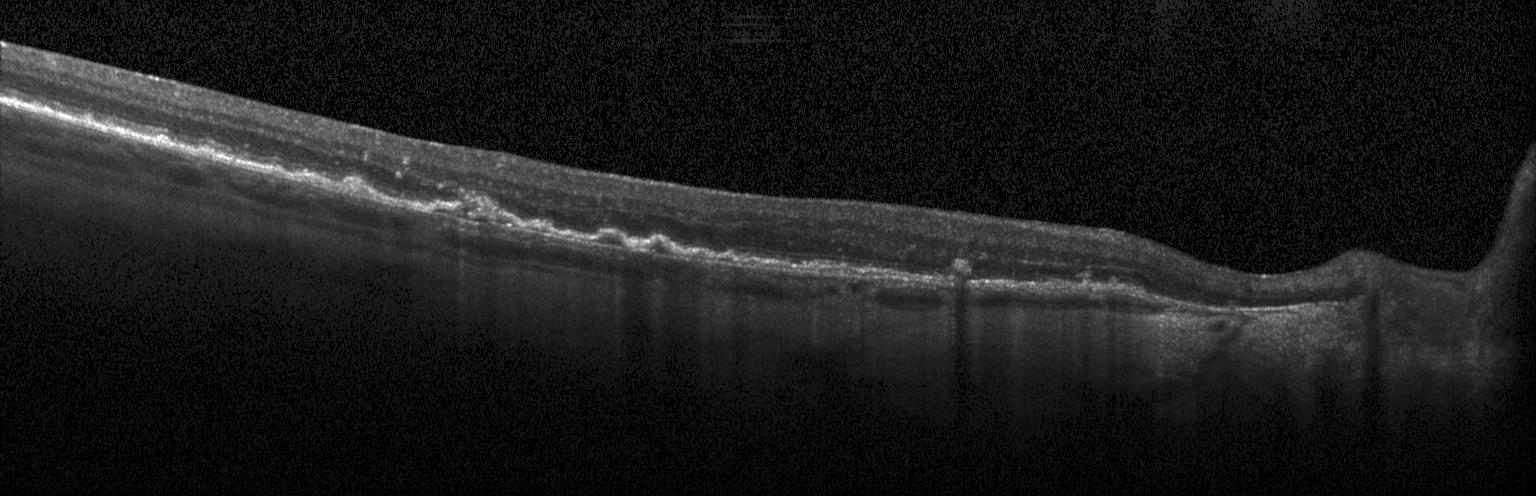
Through the macula · retinal OCT B-scan · SD-OCT · Heidelberg Spectralis.
Impression: CNV.